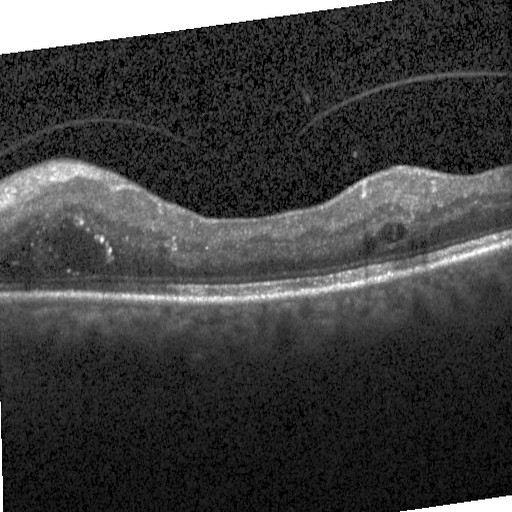 Retinal OCT cross-section, centered on the fovea
Dx: DME.